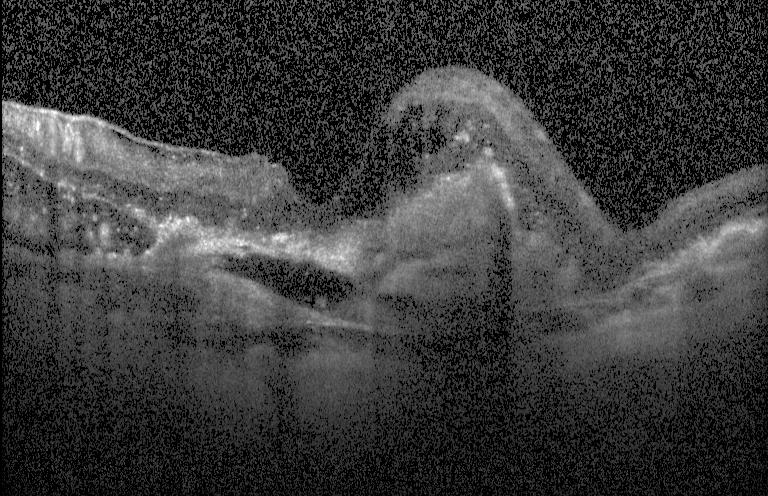 Optical coherence tomography scan. Spectral-domain OCT. Horizontal scan through the fovea. Heidelberg Spectralis.
OCT finding: a choroidal neovascular membrane.